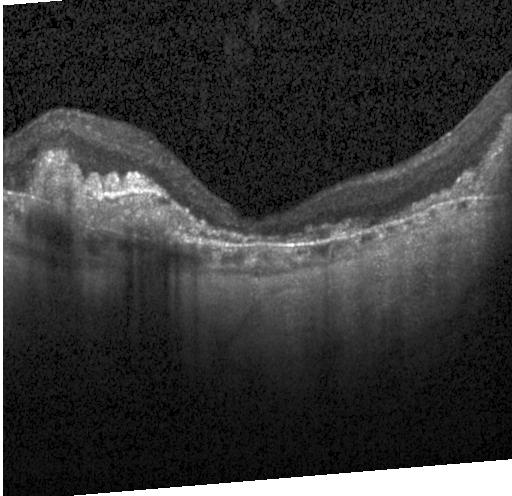
Instrument: Heidelberg Spectralis · retinal OCT cross-section · horizontal scan through the fovea · spectral-domain optical coherence tomography.
This B-scan demonstrates a choroidal neovascular membrane.